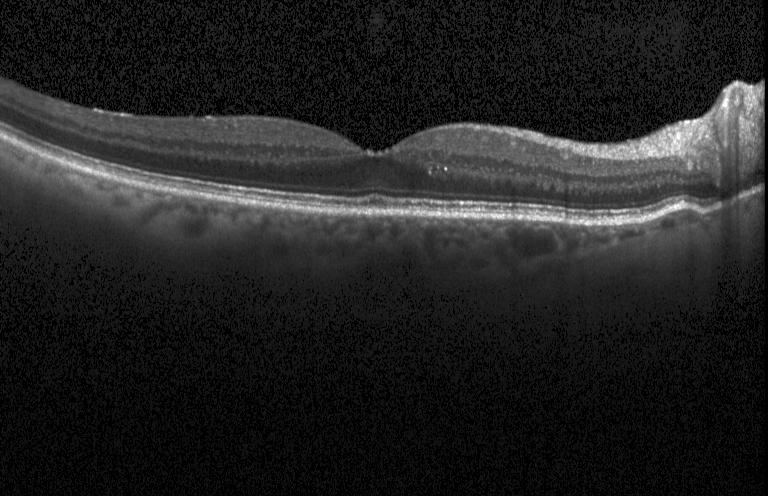 Instrument: Heidelberg Spectralis. Spectral-domain optical coherence tomography. Retinal OCT cross-section.
No evidence of choroidal neovascularization, diabetic macular edema, or drusen.